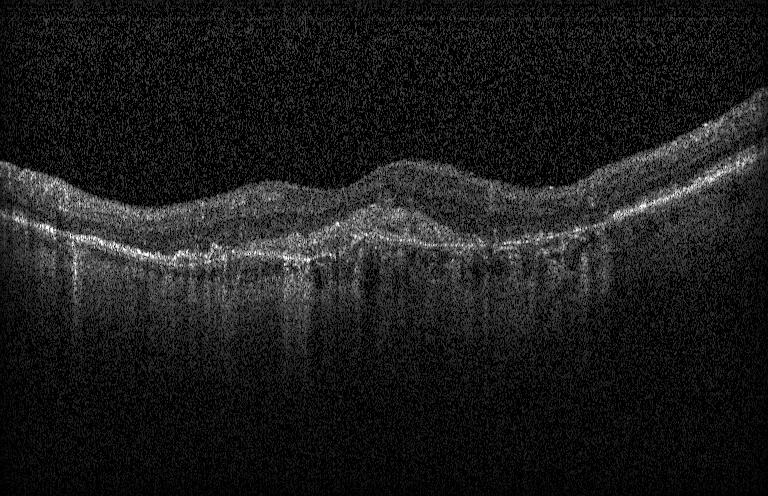
Retinal OCT cross-section. Acquired on a Heidelberg Spectralis. Centered on the fovea — Finding: a choroidal neovascular membrane.